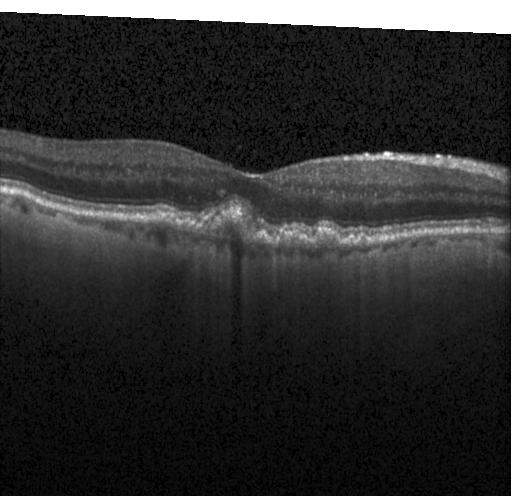 Optical coherence tomography B-scan; macular scan; instrument: Heidelberg Spectralis. Assessment: multiple drusen.